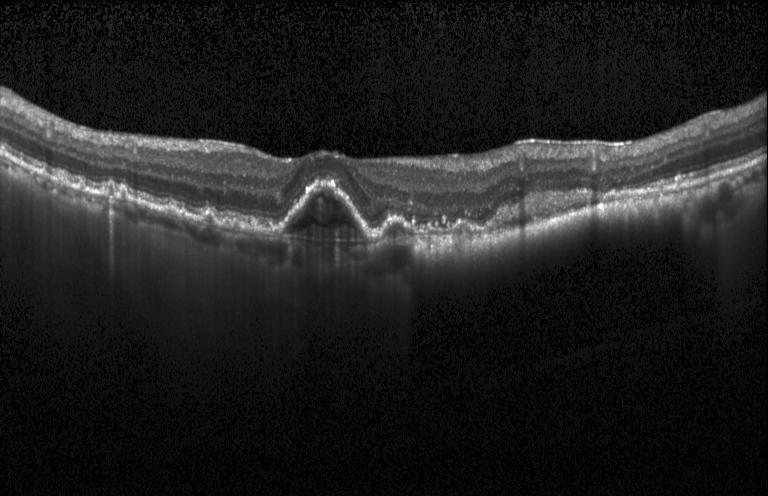

SD-OCT; OCT line scan; fovea-centered
OCT finding: a choroidal neovascular membrane.